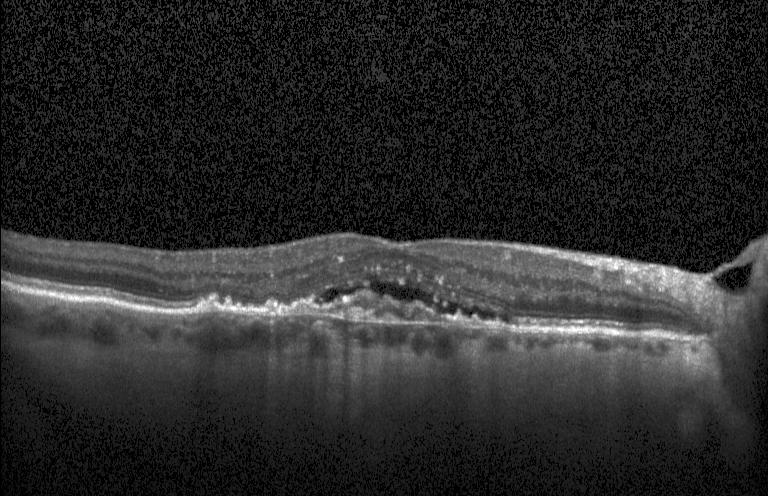
Retinal OCT cross-section showing choroidal neovascularization (CNV).